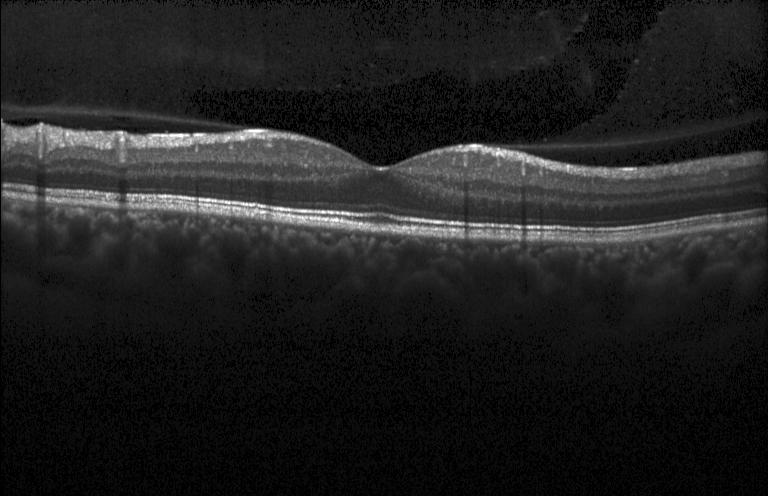

Spectral-domain OCT, Heidelberg Spectralis, OCT B-scan, through the macula — The scan shows no evidence of CNV, DME, or drusen.